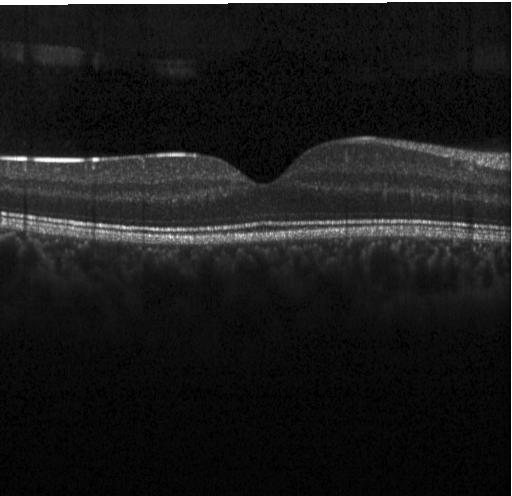 Macular scan · optical coherence tomography scan · acquired on a Heidelberg Spectralis · spectral-domain optical coherence tomography — Finding: no choroidal neovascularization, diabetic macular edema, or drusen.